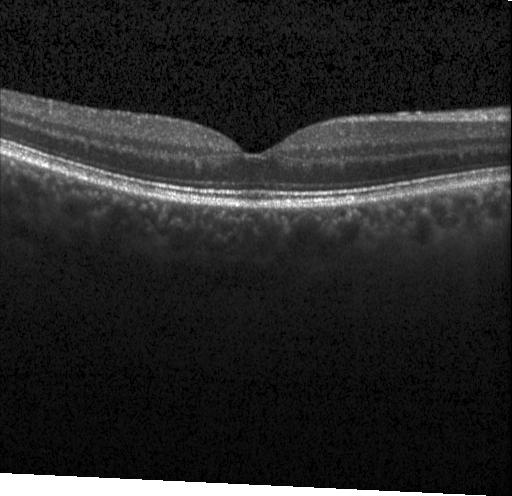

Retinal OCT B-scan. Diagnosis: no choroidal neovascularization, no diabetic macular edema, and no drusen.